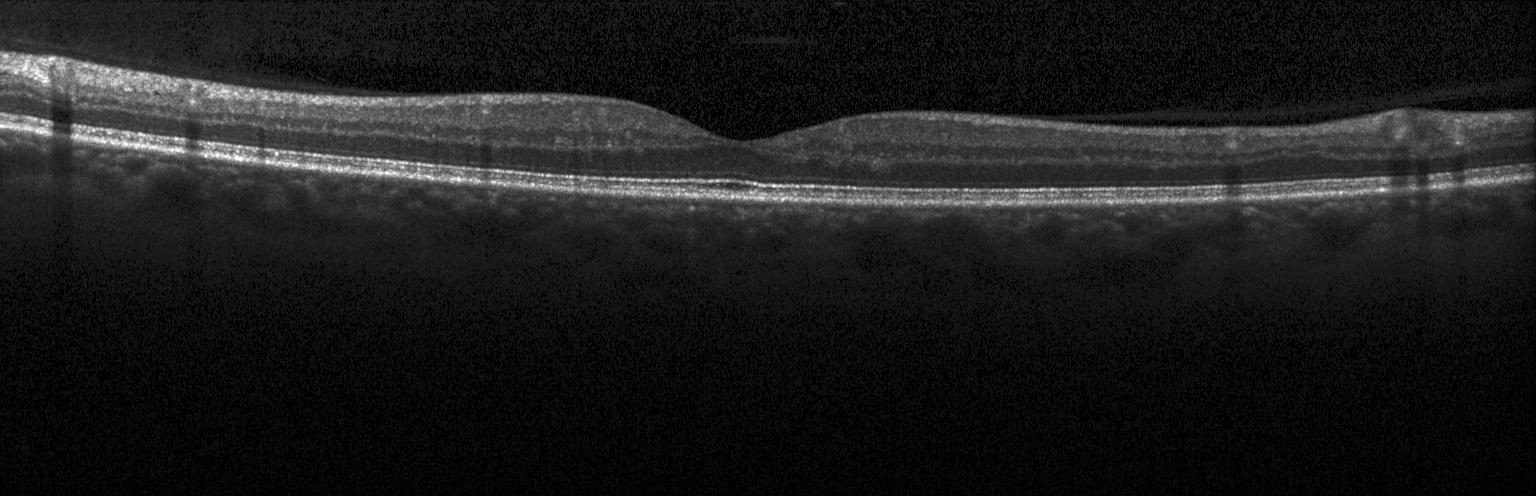 SD-OCT · through the macula · instrument: Heidelberg Spectralis · OCT line scan. Dx: no choroidal neovascularization, diabetic macular edema, or drusen.